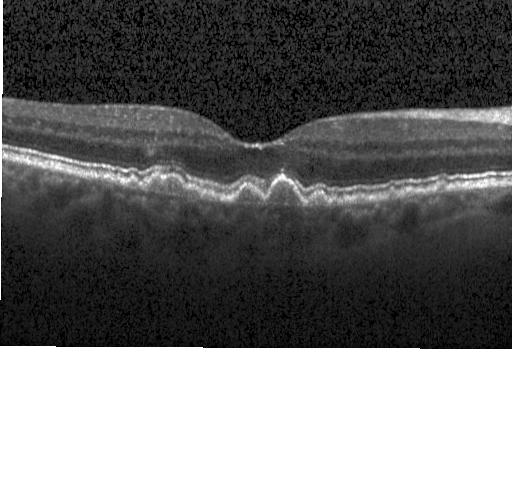
Fovea-centered. Optical coherence tomography scan — OCT finding: multiple drusen.